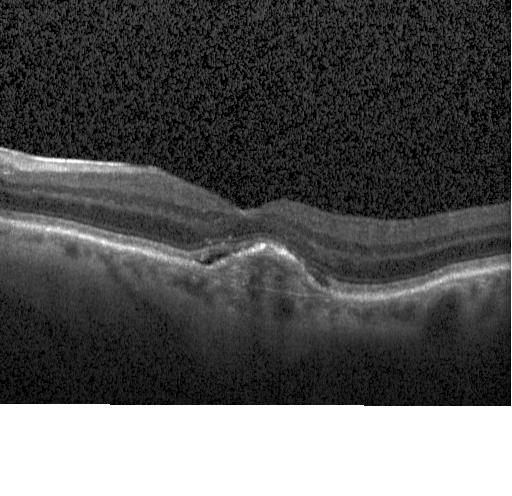
Heidelberg Spectralis OCT system, OCT line scan — Diagnosis: a choroidal neovascular membrane.